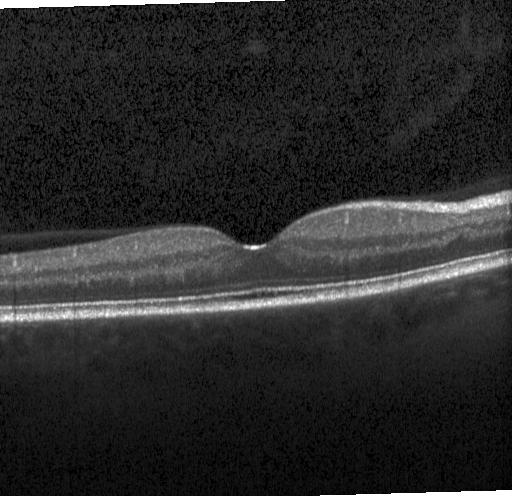

Diagnosis: no choroidal neovascularization, diabetic macular edema, or drusen.